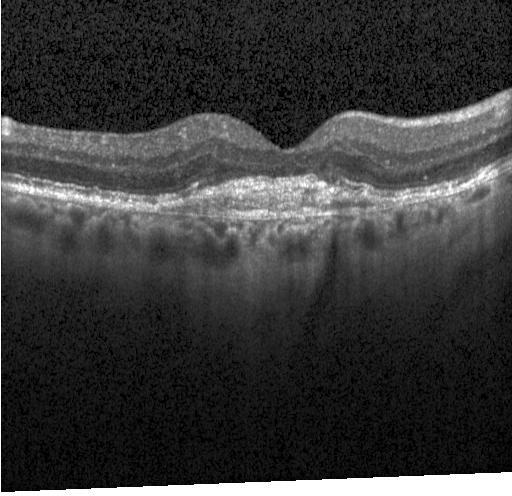 Finding: choroidal neovascularization (CNV).